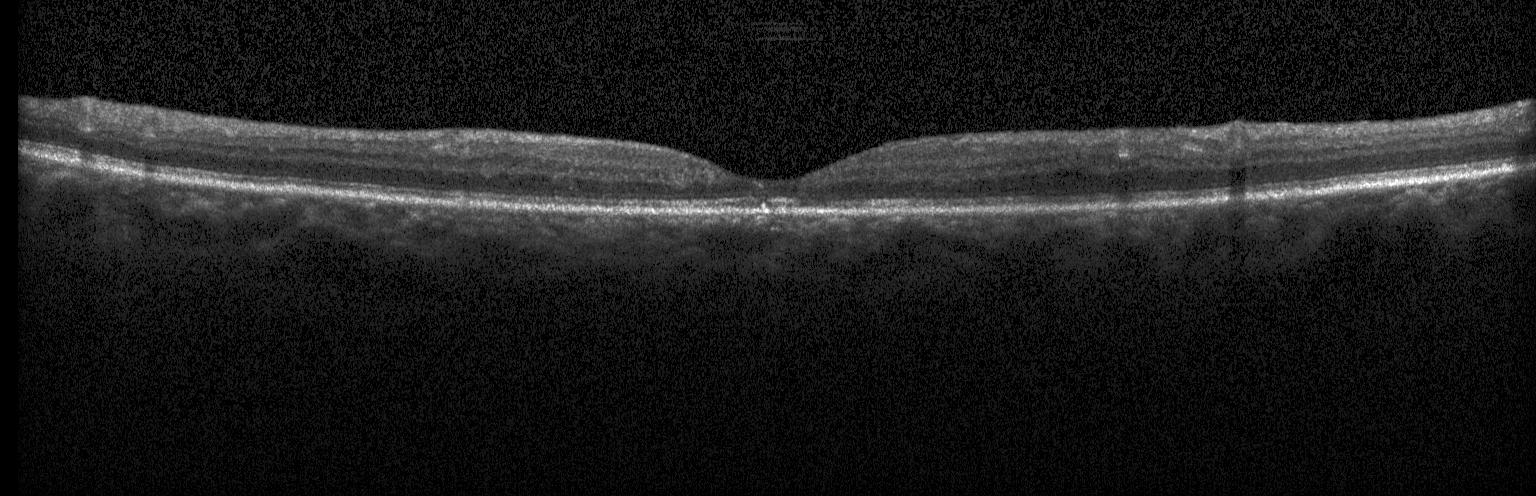

Retinal OCT B-scan, fovea-centered. Impression: no CNV, DME, or drusen.